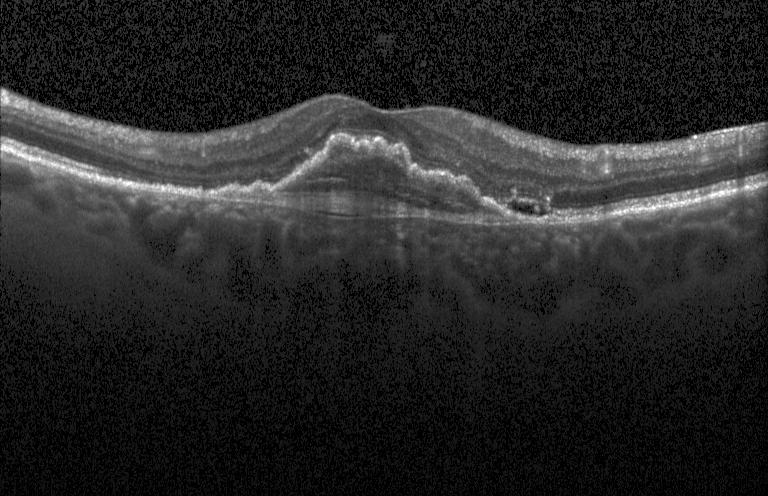

Optical coherence tomography B-scan; instrument: Heidelberg Spectralis; horizontal scan through the fovea.
Diagnosis: a choroidal neovascular membrane.